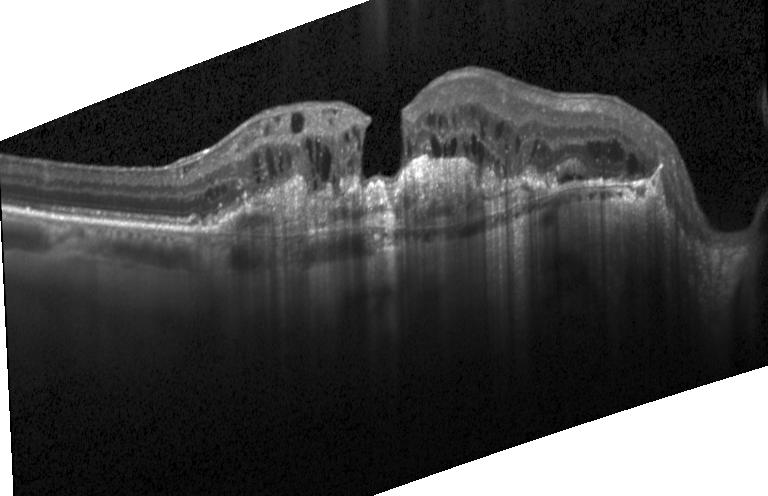
Retinal OCT B-scan · horizontal scan through the fovea — This B-scan demonstrates a choroidal neovascular membrane.